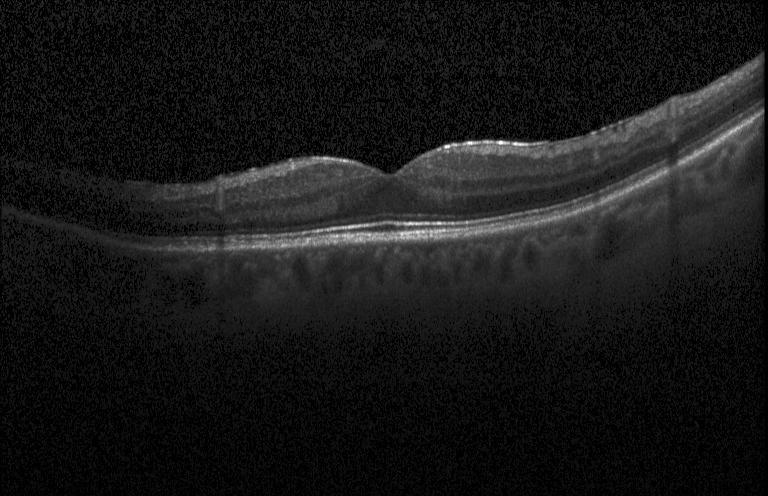
OCT finding: no choroidal neovascularization, diabetic macular edema, or drusen.